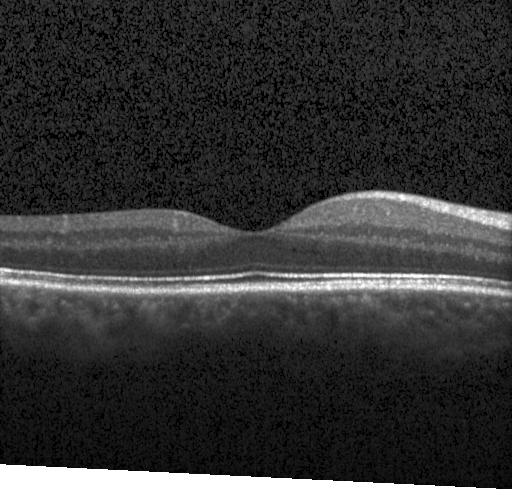 Optical coherence tomography scan.
Assessment: no choroidal neovascularization, no diabetic macular edema, and no drusen.